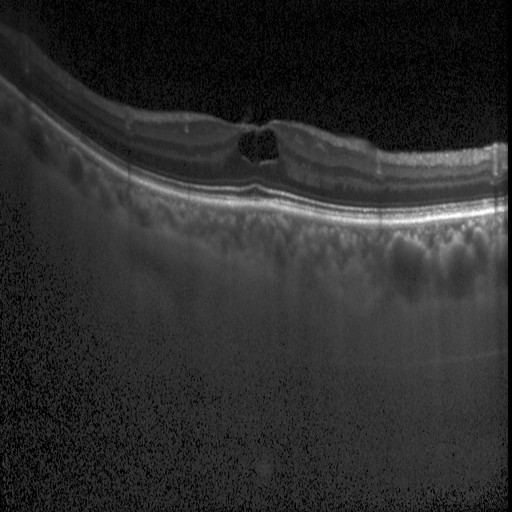

Optical coherence tomography B-scan · through the macula · instrument: Heidelberg Spectralis
Diagnosis: DME.